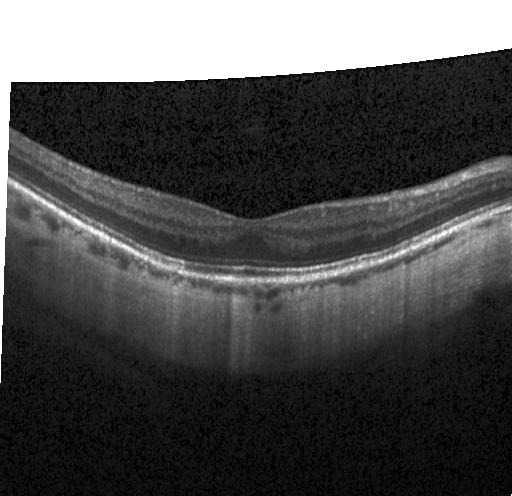
Retinal OCT cross-section, acquired on a Heidelberg Spectralis
Impression: no evidence of choroidal neovascularization, diabetic macular edema, or drusen.